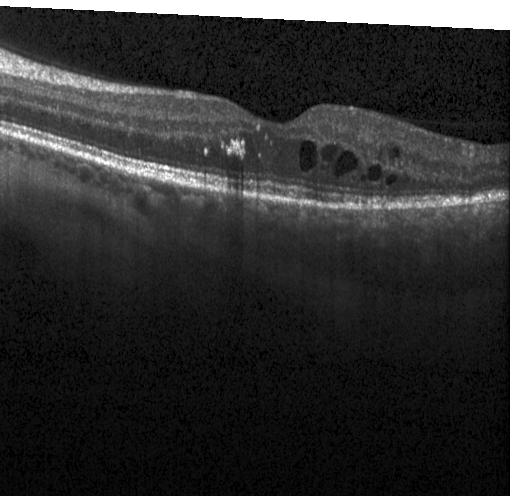 Optical coherence tomography scan — Finding: diabetic macular edema.